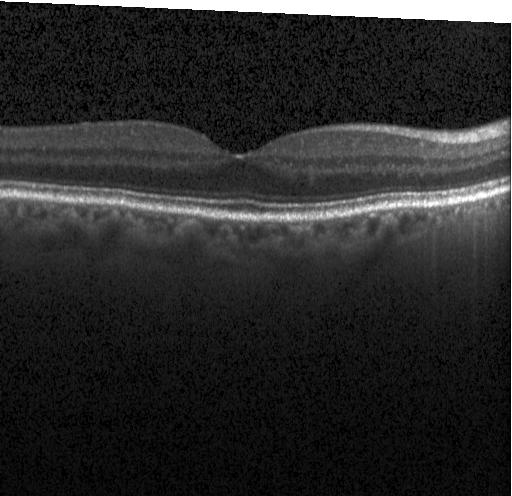 Heidelberg Spectralis; spectral-domain OCT; optical coherence tomography B-scan. Impression: no choroidal neovascularization, diabetic macular edema, or drusen.